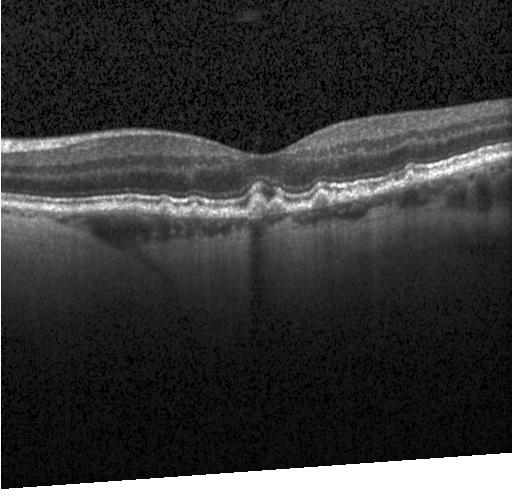 Spectral-domain OCT B-scan: drusen.